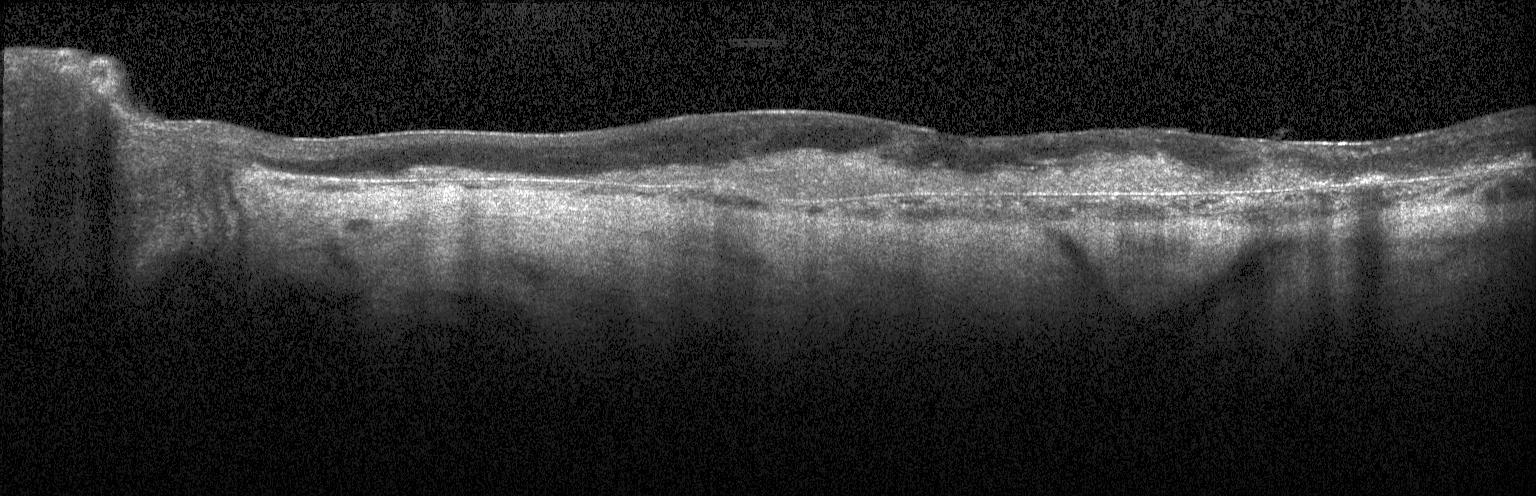 Retinal OCT cross-section showing a choroidal neovascular membrane.